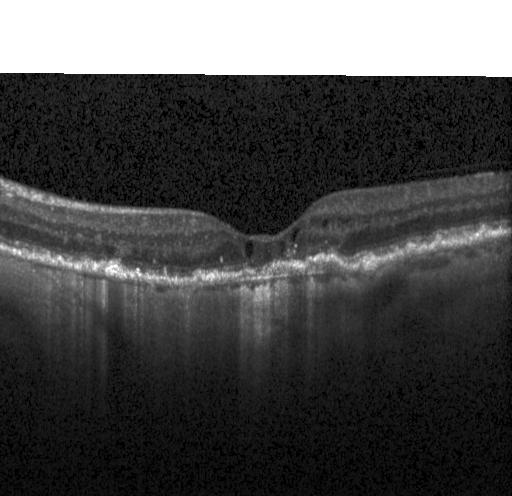
OCT finding: choroidal neovascularization (CNV).